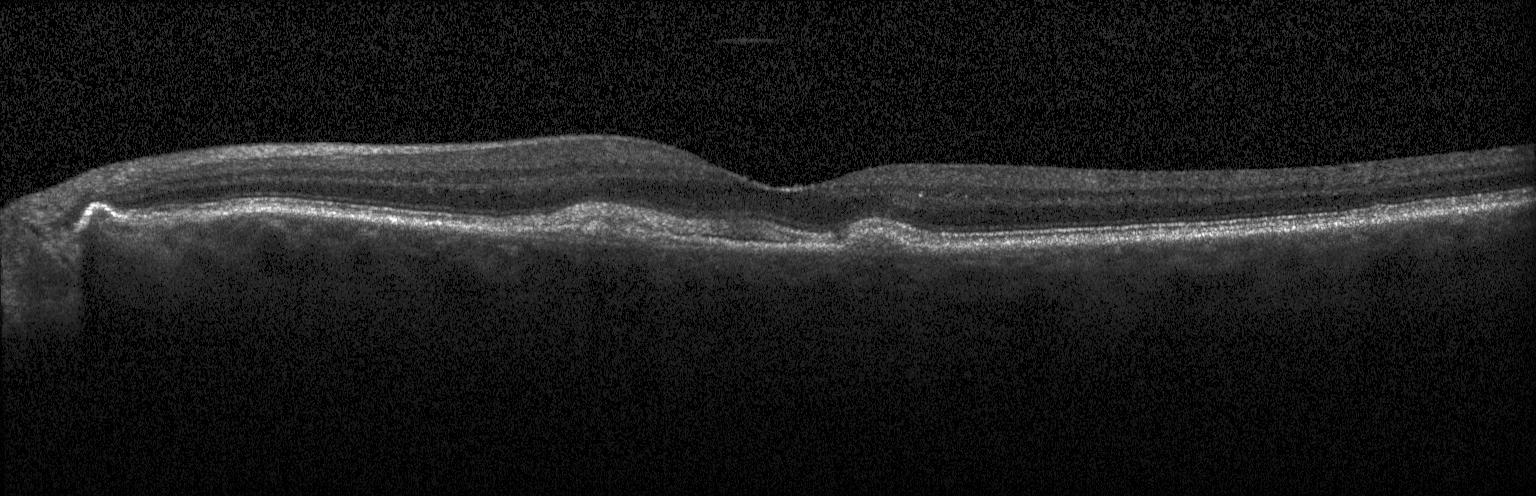 SD-OCT; horizontal scan through the fovea; optical coherence tomography B-scan.
Impression: a choroidal neovascular membrane.